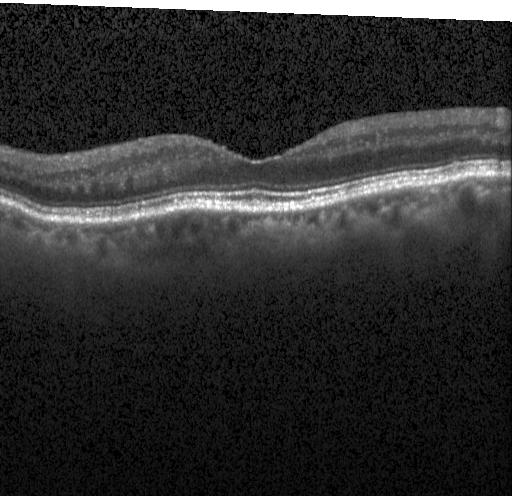 Diagnosis: no evidence of CNV, DME, or drusen.